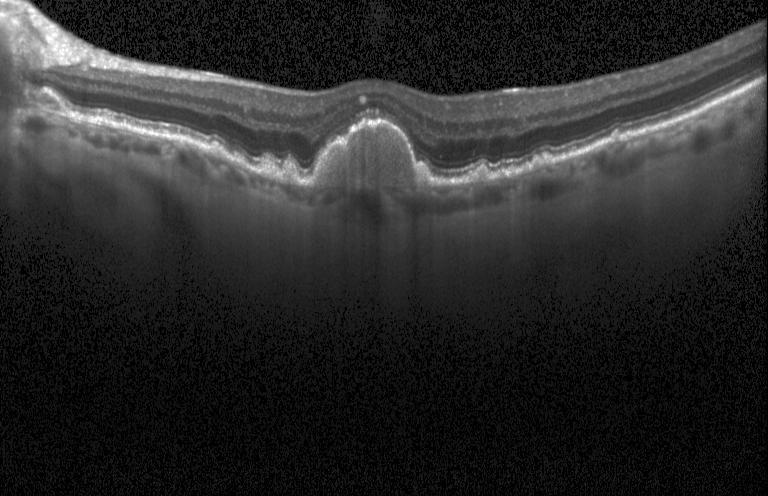 Finding: drusen.